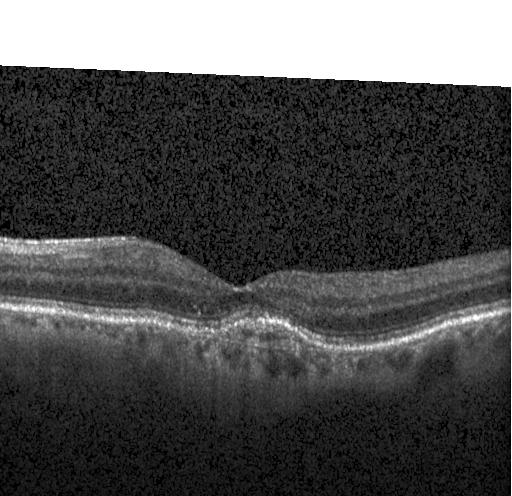
Retinal OCT B-scan.
OCT finding: choroidal neovascularization.